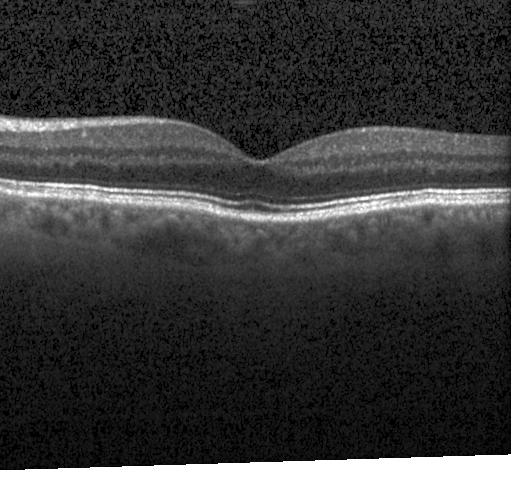

OCT line scan — Diagnosis: no choroidal neovascularization, diabetic macular edema, or drusen.